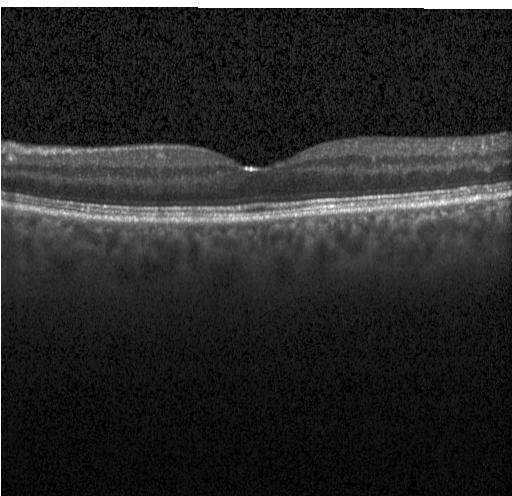 Diagnosis: no evidence of choroidal neovascularization, diabetic macular edema, or drusen.